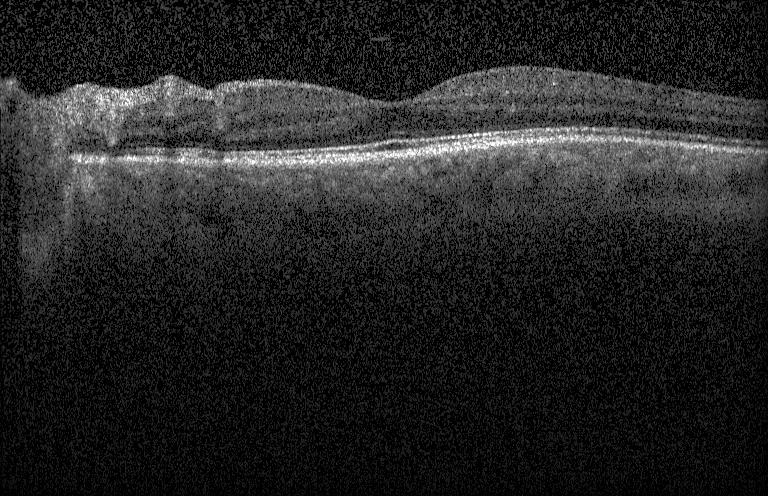
Neither choroidal neovascularization, diabetic macular edema, nor drusen.